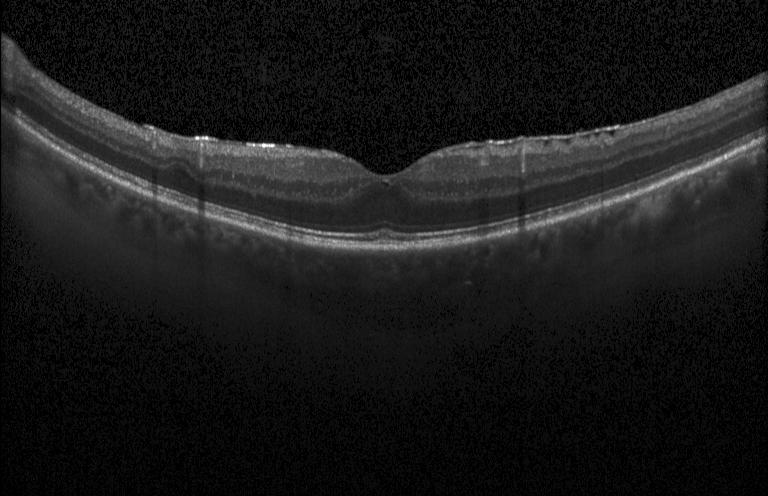
Assessment: no choroidal neovascularization, no diabetic macular edema, and no drusen.